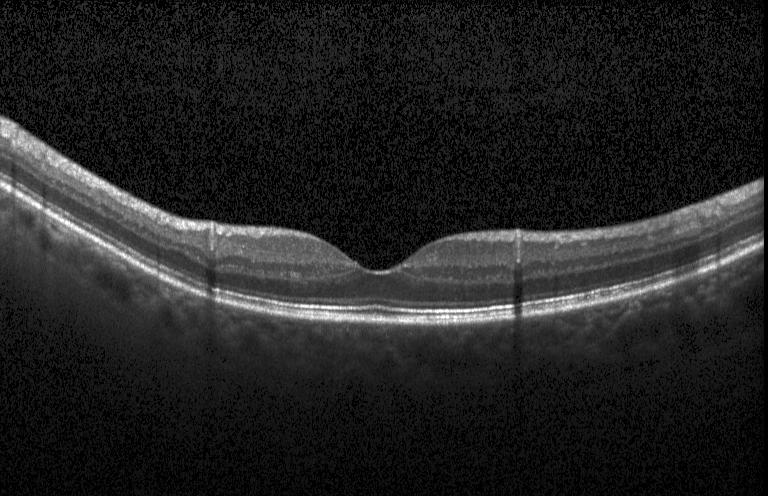
Retinal OCT B-scan; SD-OCT. The scan shows neither CNV, DME, nor drusen.